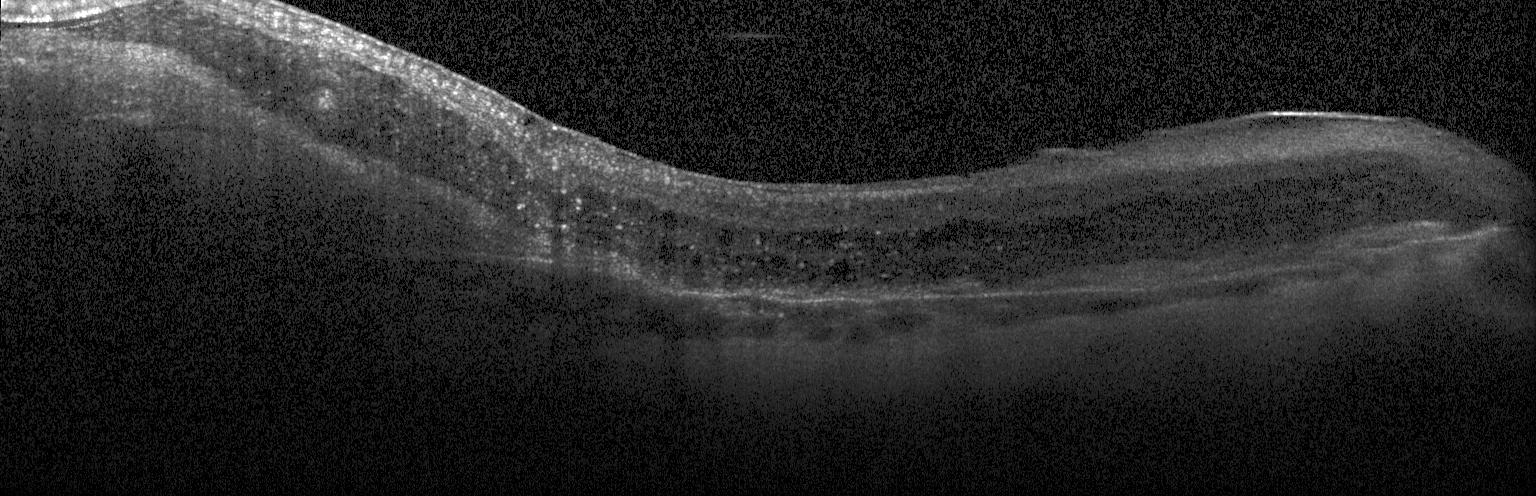
Optical coherence tomography B-scan; spectral-domain OCT
This B-scan demonstrates choroidal neovascularization.